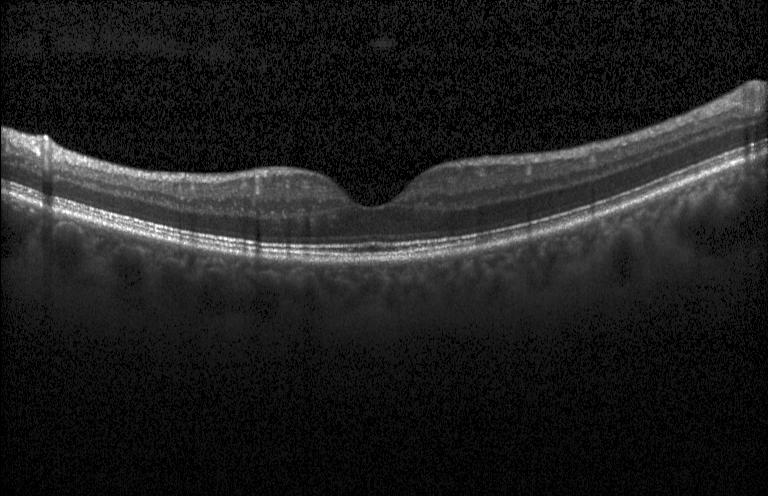

Heidelberg Spectralis · spectral-domain OCT · optical coherence tomography scan. Impression: no CNV, no DME, and no drusen.